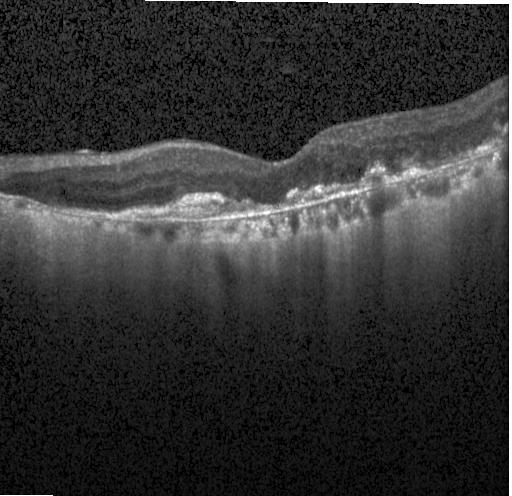
OCT B-scan showing a choroidal neovascular membrane.